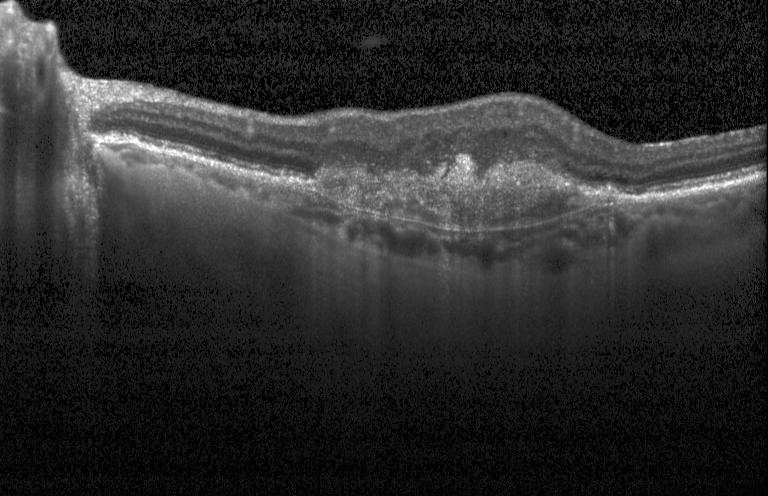
Diagnosis: CNV.